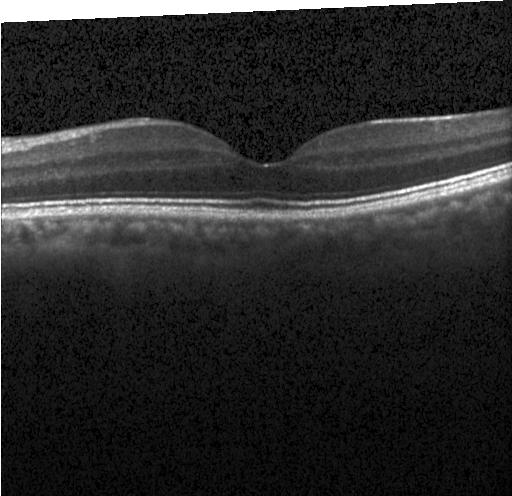 Fovea-centered · OCT line scan · acquired on a Heidelberg Spectralis · spectral-domain OCT — Assessment: no choroidal neovascularization, diabetic macular edema, or drusen.